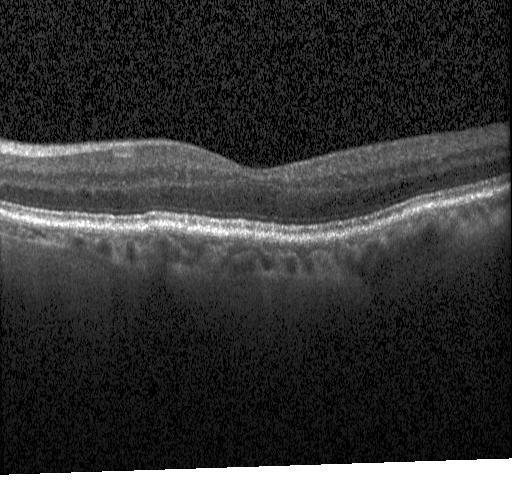

Impression: no evidence of CNV, DME, or drusen.